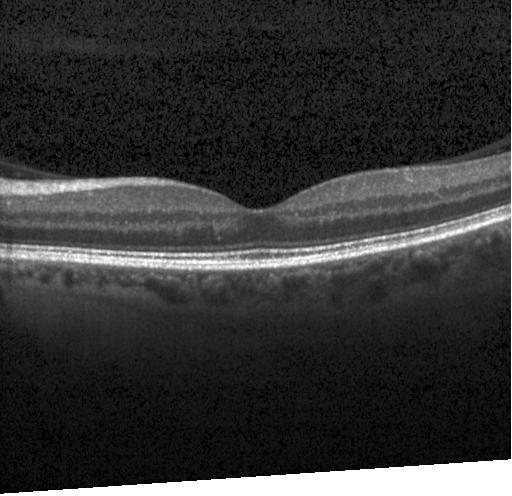 Optical coherence tomography B-scan.
Impression: neither CNV, DME, nor drusen.